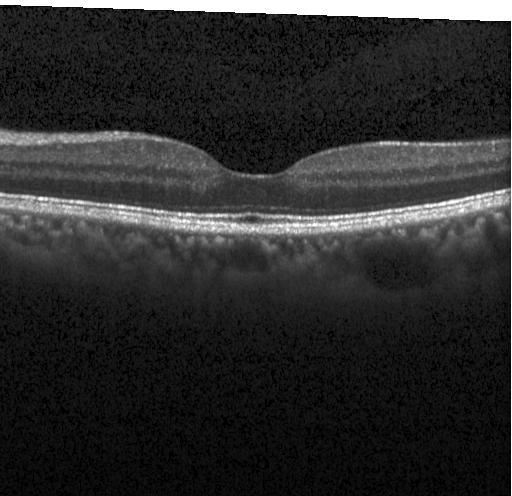

Through the macula · OCT line scan
OCT finding: neither choroidal neovascularization, diabetic macular edema, nor drusen.